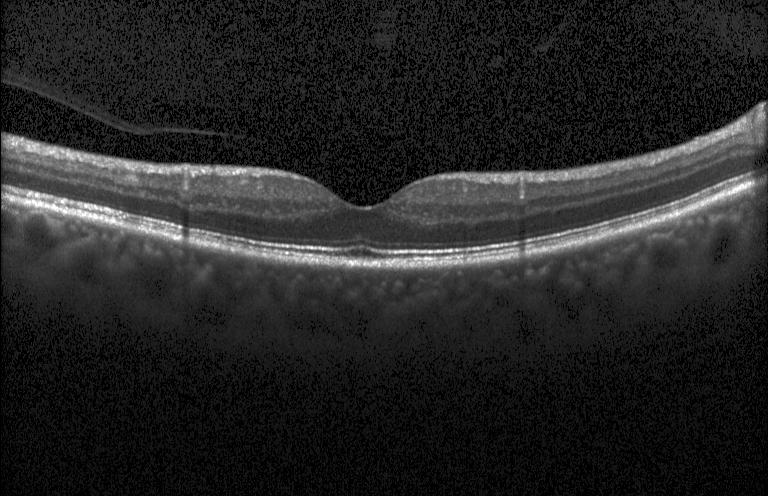
Centered on the fovea; optical coherence tomography scan; SD-OCT.
Neither choroidal neovascularization, diabetic macular edema, nor drusen.